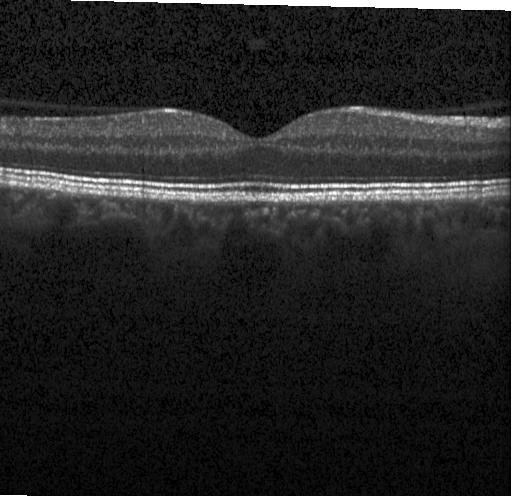

Finding: no choroidal neovascularization, diabetic macular edema, or drusen.